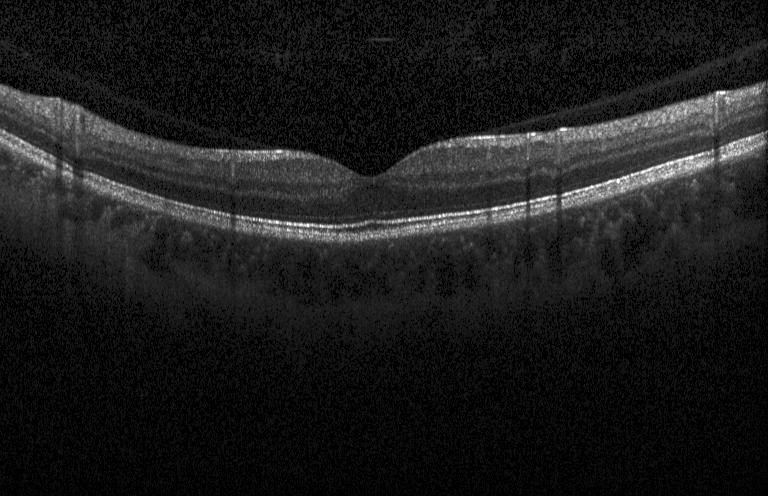
The scan shows no choroidal neovascularization, no diabetic macular edema, and no drusen.